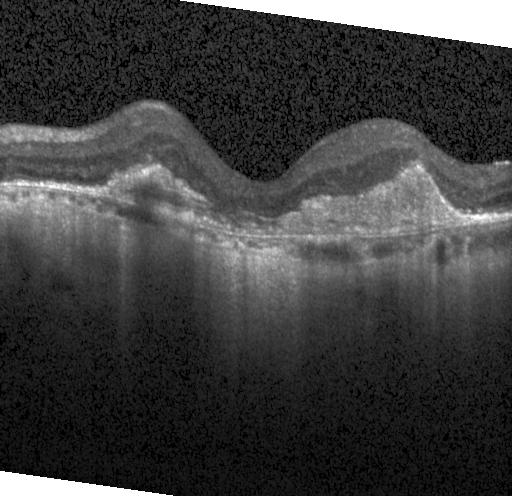

The scan shows CNV.